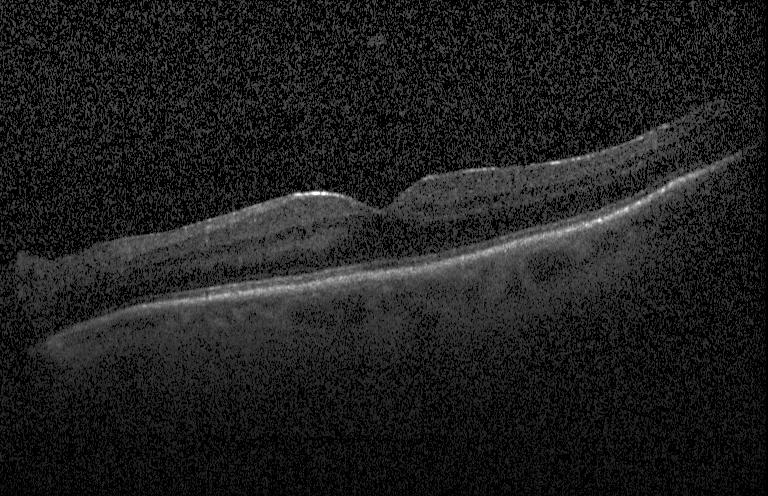
Optical coherence tomography scan, Heidelberg Spectralis, SD-OCT, macular scan — The scan shows no choroidal neovascularization, diabetic macular edema, or drusen.